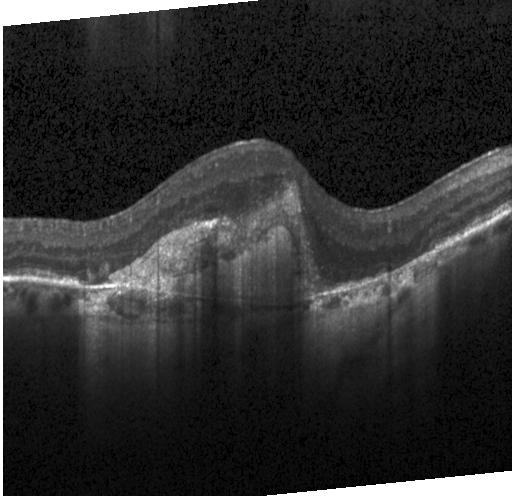
Optical coherence tomography B-scan. Spectral-domain OCT. Through the macula.
CNV.